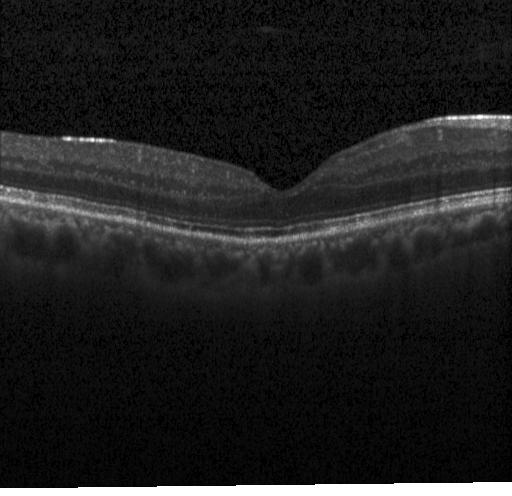

Dx: neither choroidal neovascularization, diabetic macular edema, nor drusen.